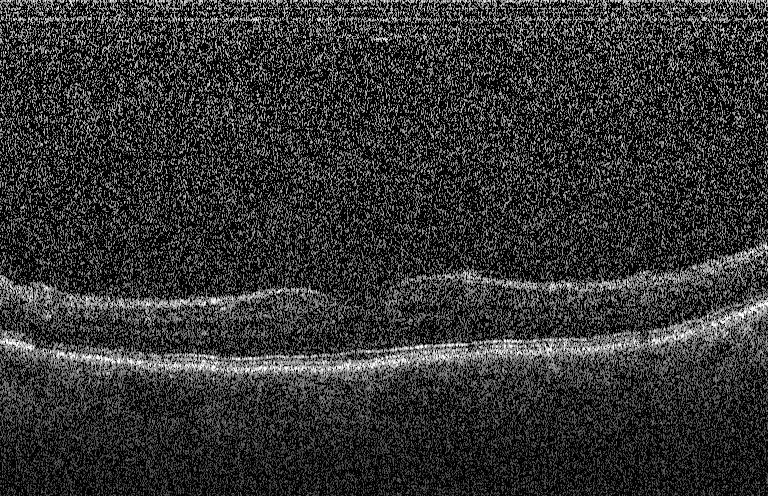
Through the macula; Heidelberg Spectralis; OCT B-scan; spectral-domain OCT.
OCT finding: no evidence of choroidal neovascularization, diabetic macular edema, or drusen.